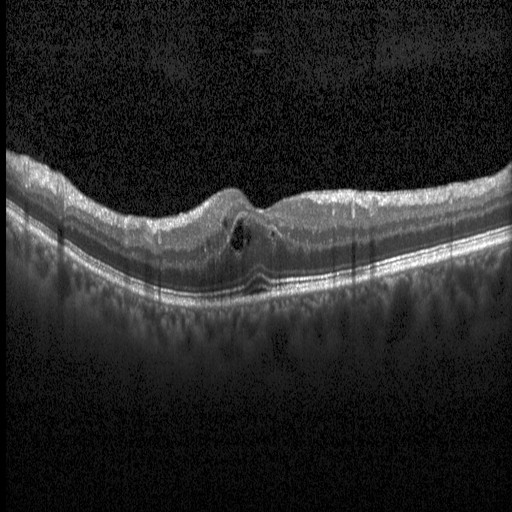
This B-scan demonstrates diabetic macular edema (DME).